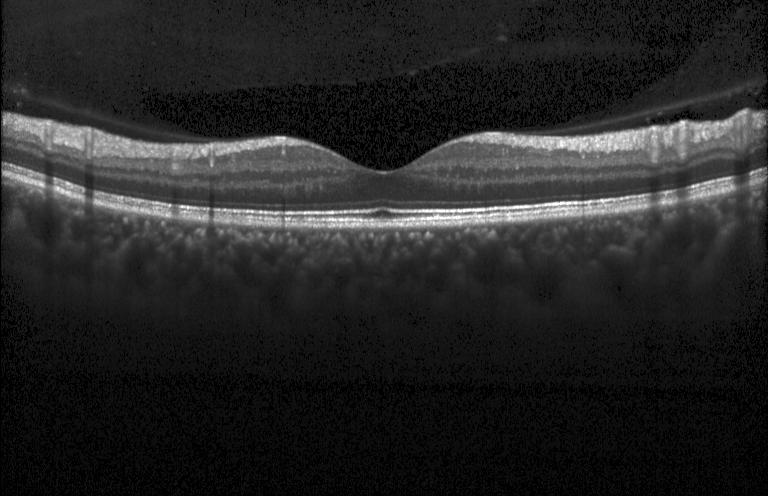
OCT scan showing no evidence of choroidal neovascularization, diabetic macular edema, or drusen.